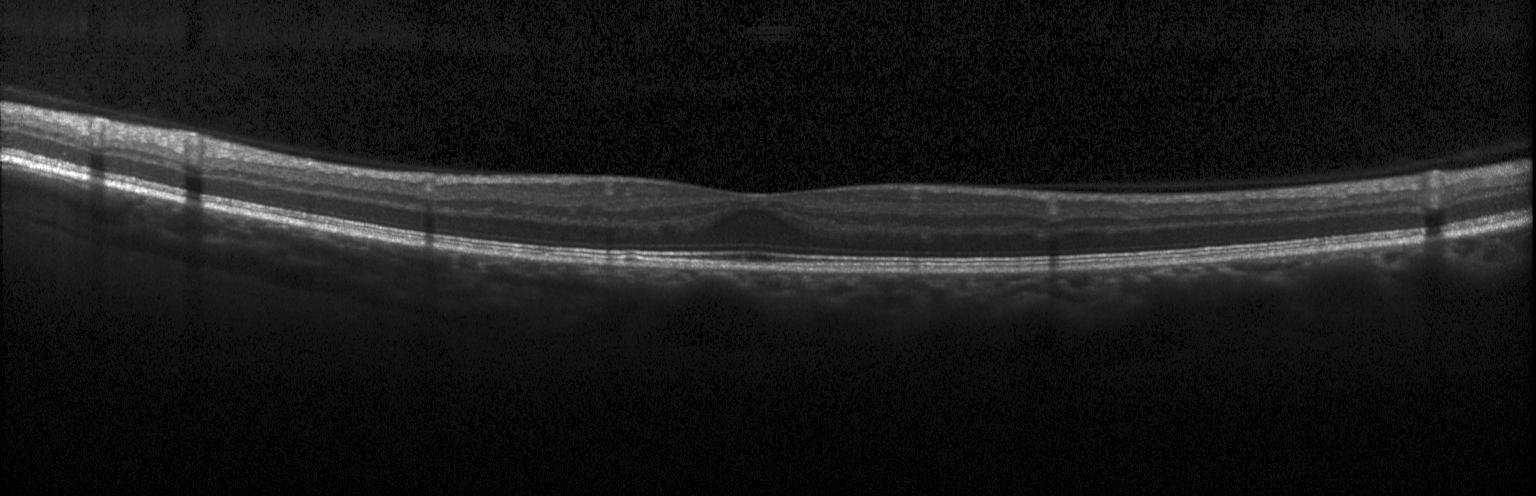
Impression: no choroidal neovascularization, diabetic macular edema, or drusen.